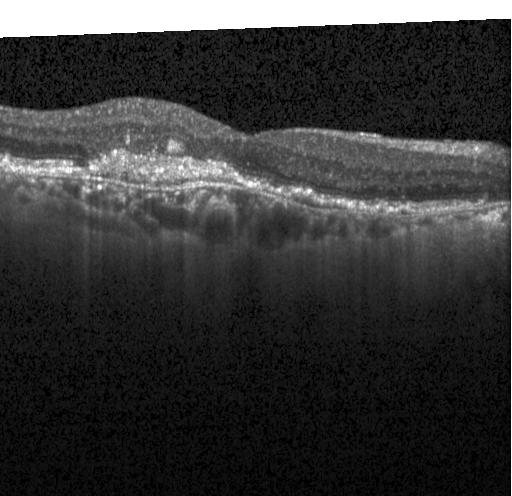

Finding: a choroidal neovascular membrane.